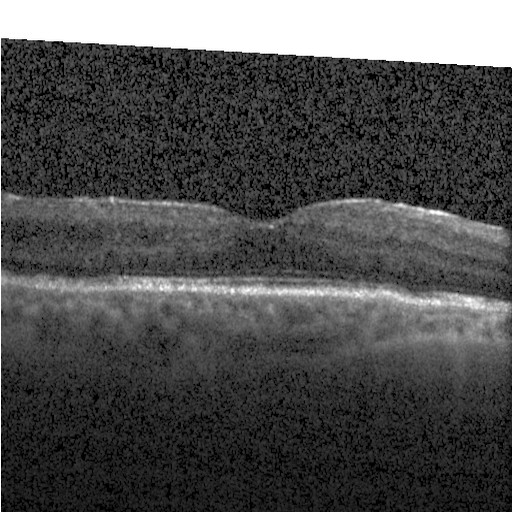 Macular scan · OCT line scan · spectral-domain OCT — The scan shows diabetic macular edema.